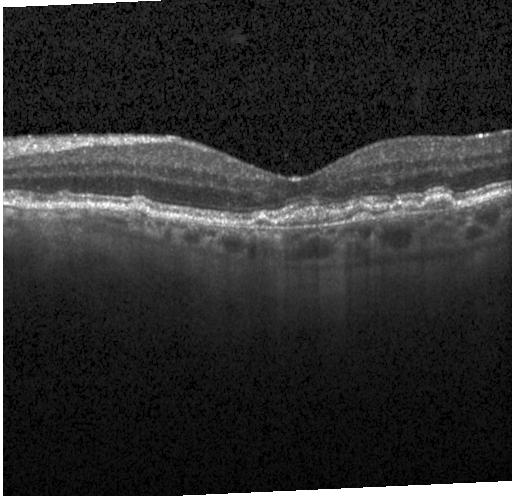

Horizontal scan through the fovea; retinal OCT B-scan.
Diagnosis: a choroidal neovascular membrane.